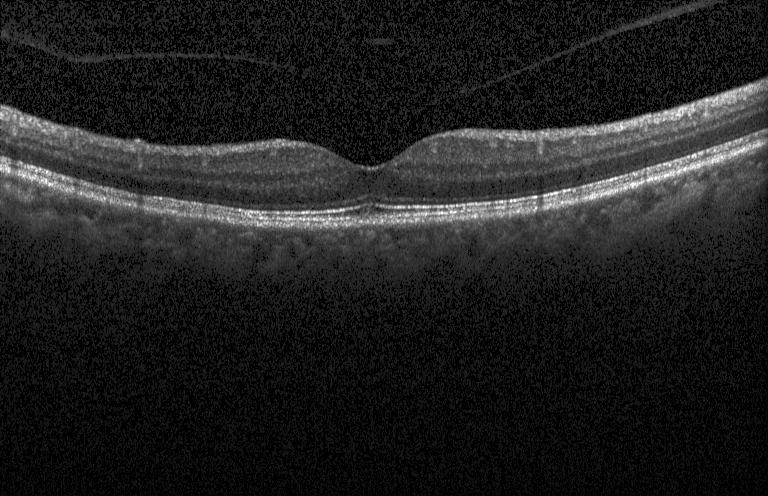
Retinal OCT B-scan. Macular scan. OCT finding: no CNV, no DME, and no drusen.